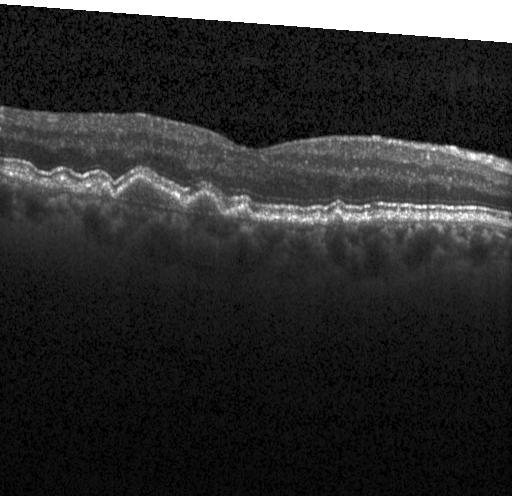

This B-scan demonstrates drusen.